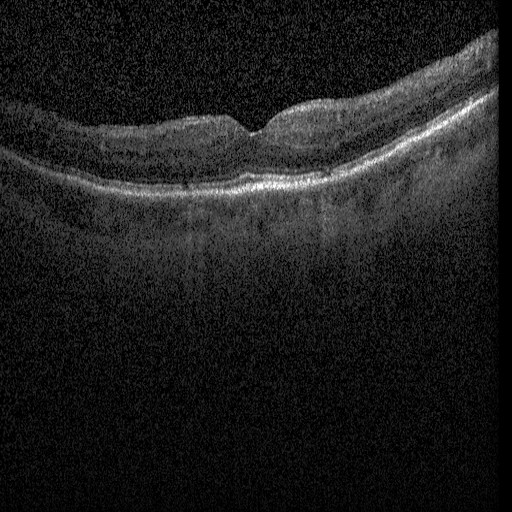
Dx: diabetic macular edema (DME).